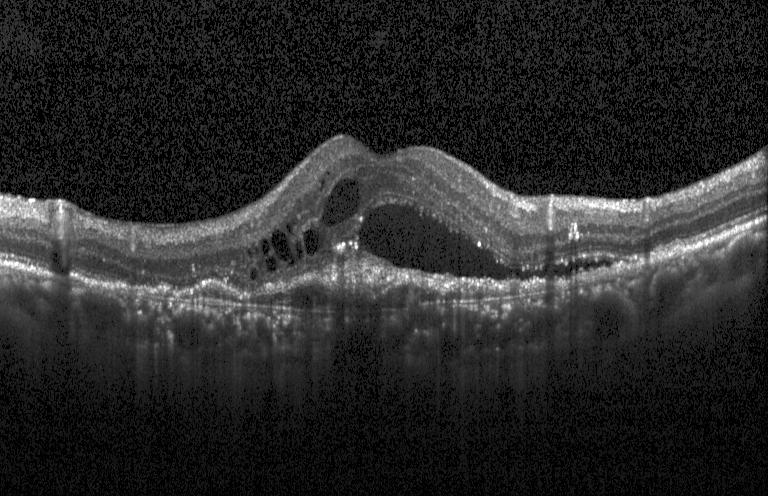

Diagnosis: a choroidal neovascular membrane.